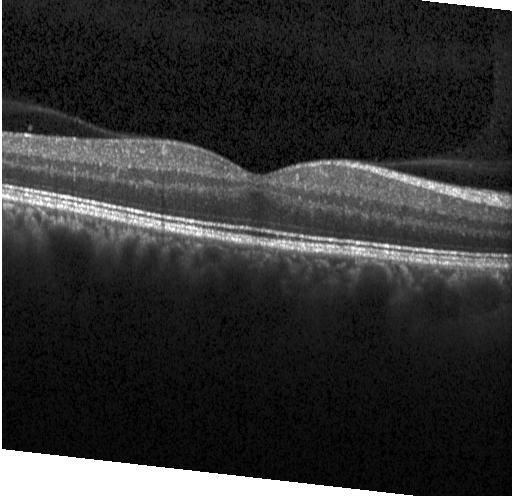 Impression: neither choroidal neovascularization, diabetic macular edema, nor drusen.